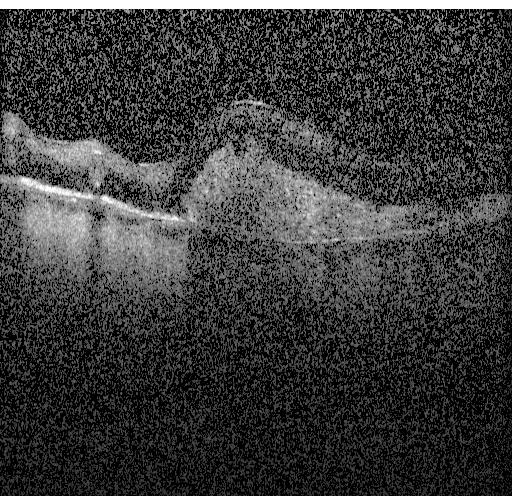

The scan shows a choroidal neovascular membrane.